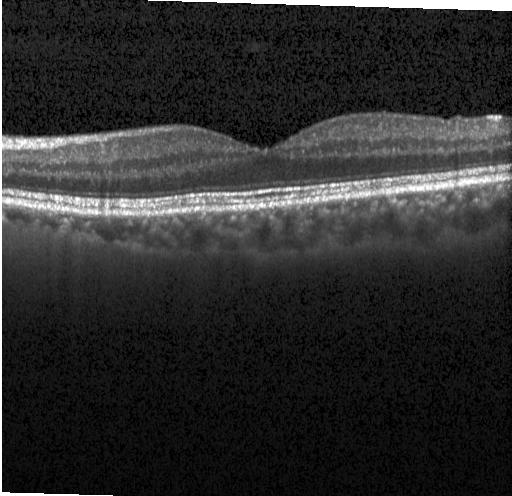 Macular OCT demonstrating no CNV, DME, or drusen.